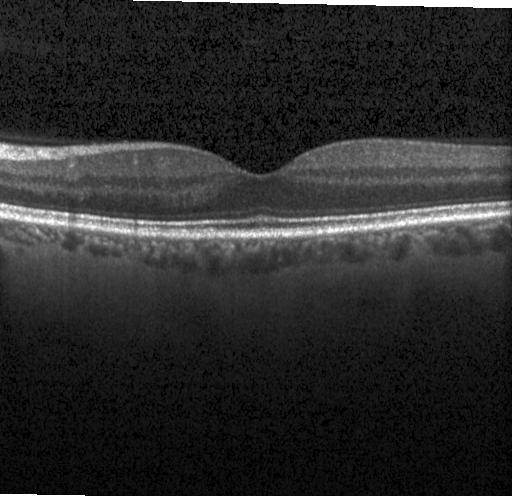

Retinal OCT cross-section.
Assessment: no CNV, no DME, and no drusen.